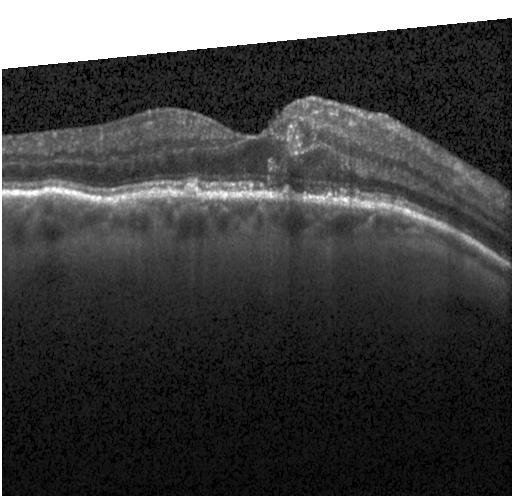

Retinal OCT cross-section; acquired on a Heidelberg Spectralis
Assessment: drusen.